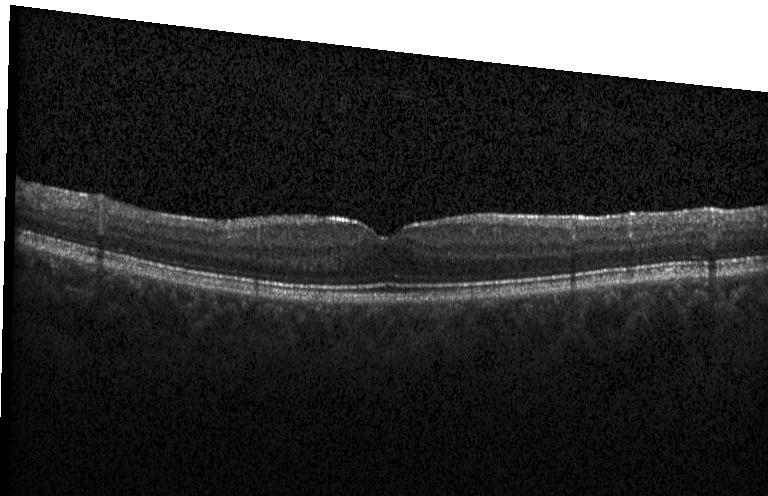

The scan shows neither choroidal neovascularization, diabetic macular edema, nor drusen.